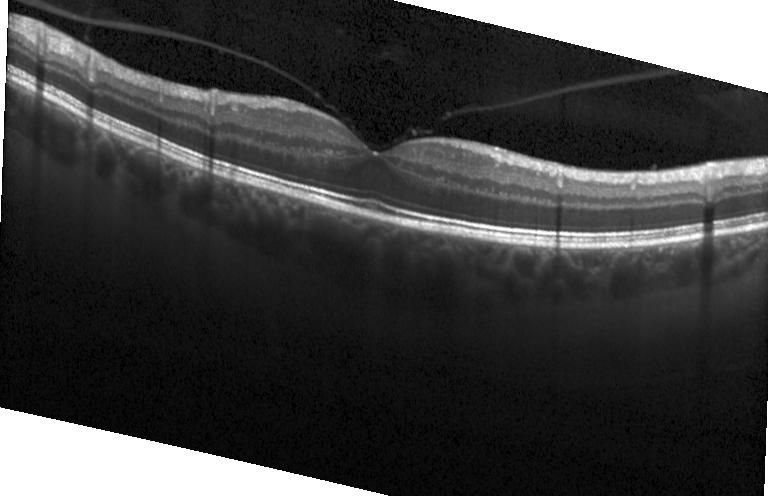
Through the macula, retinal OCT cross-section, acquired on a Heidelberg Spectralis
Assessment: no choroidal neovascularization, diabetic macular edema, or drusen.